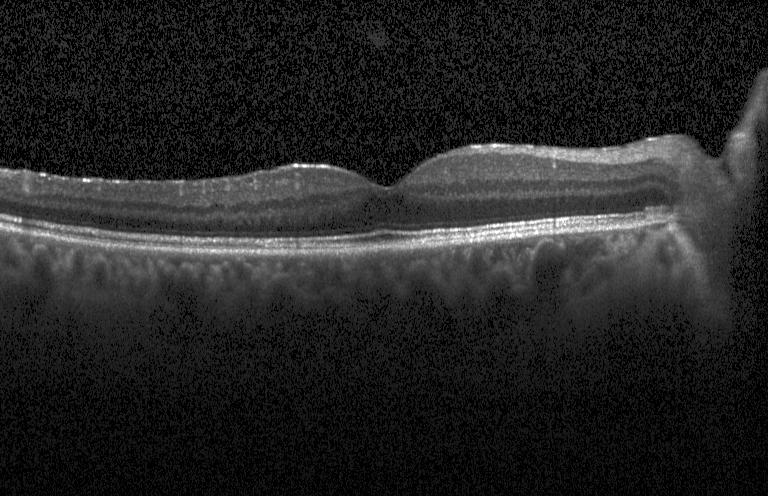 OCT B-scan. Impression: no evidence of CNV, DME, or drusen.